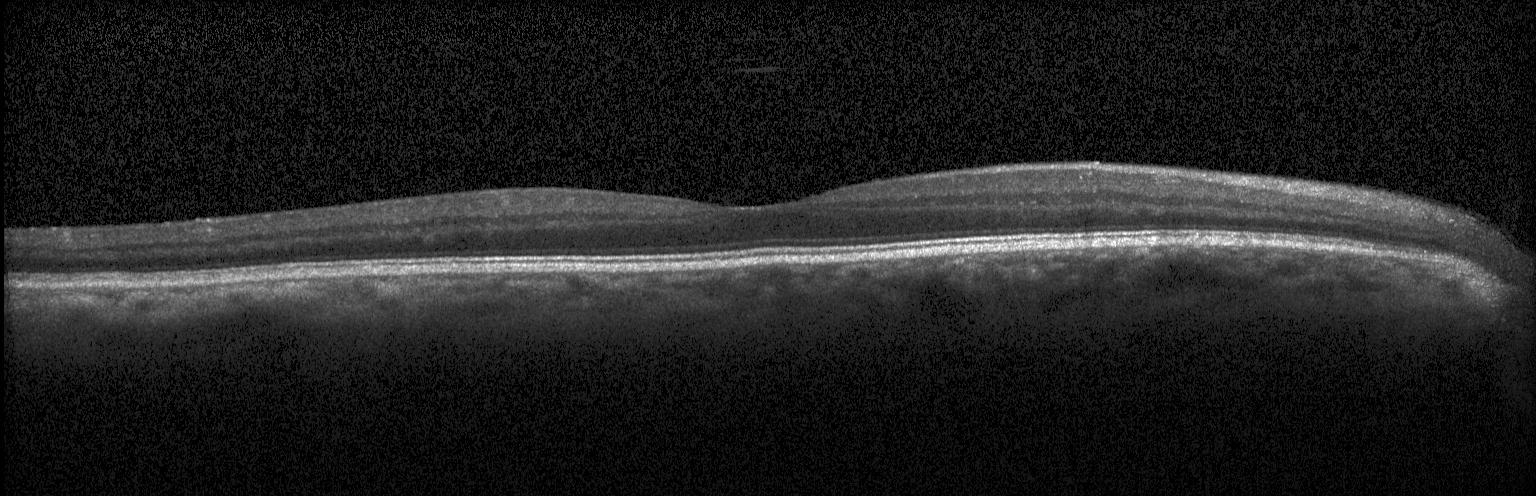 Finding: no evidence of choroidal neovascularization, diabetic macular edema, or drusen.